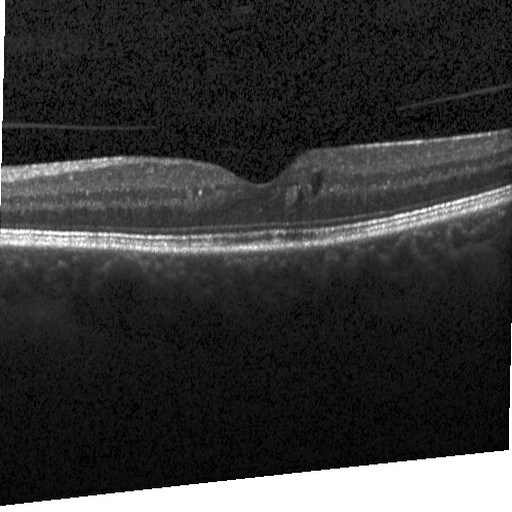
Through the macula, optical coherence tomography scan, spectral-domain optical coherence tomography
Dx: diabetic macular edema (DME).